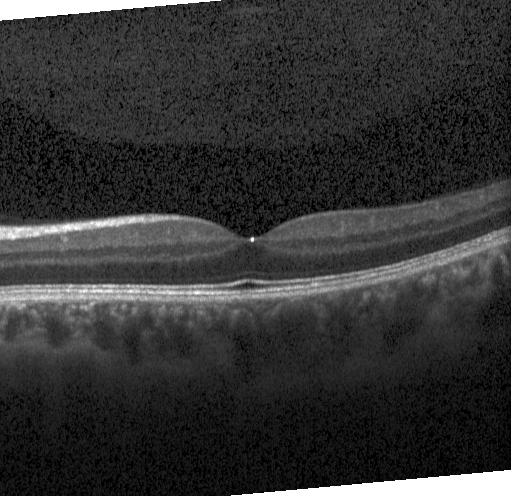
OCT line scan. Heidelberg Spectralis.
Impression: neither choroidal neovascularization, diabetic macular edema, nor drusen.